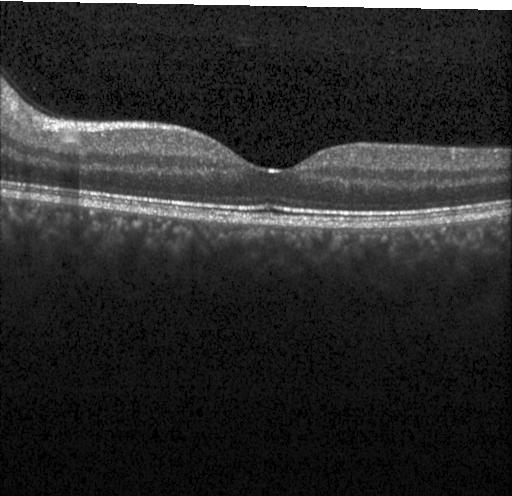

Dx: no evidence of choroidal neovascularization, diabetic macular edema, or drusen.